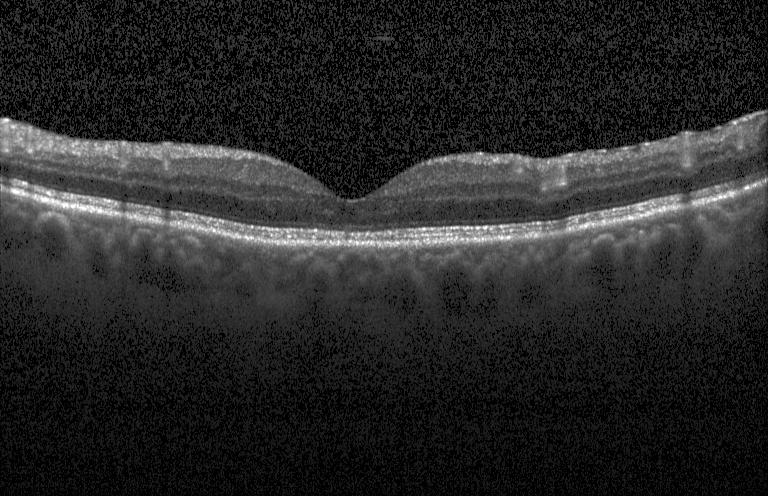 OCT scan showing no CNV, no DME, and no drusen.